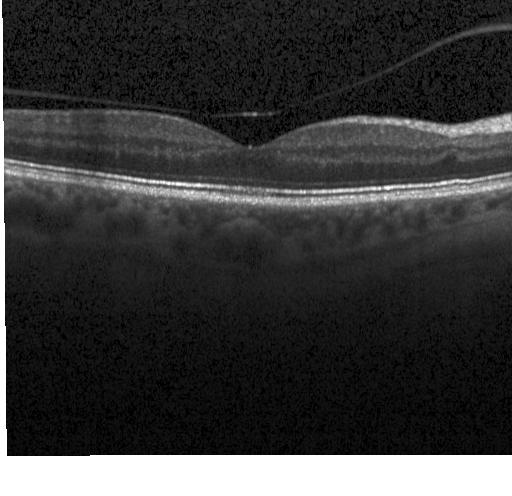 Macular OCT: no evidence of choroidal neovascularization, diabetic macular edema, or drusen.